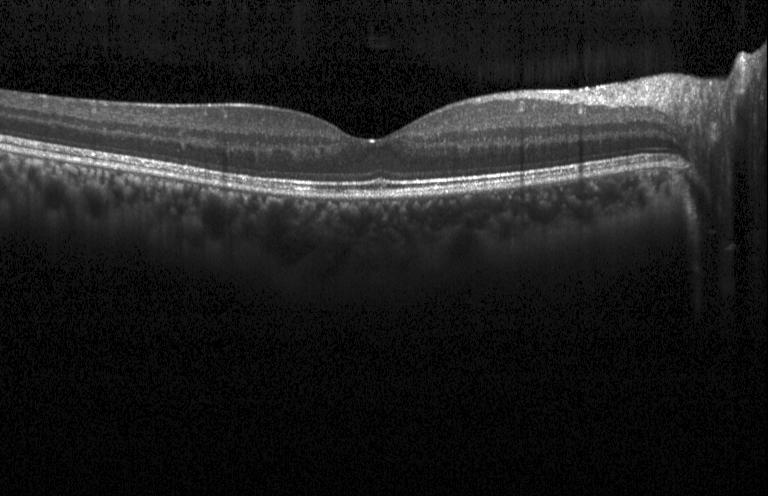
Macular scan · instrument: Heidelberg Spectralis · SD-OCT · optical coherence tomography B-scan.
Diagnosis: no choroidal neovascularization, diabetic macular edema, or drusen.